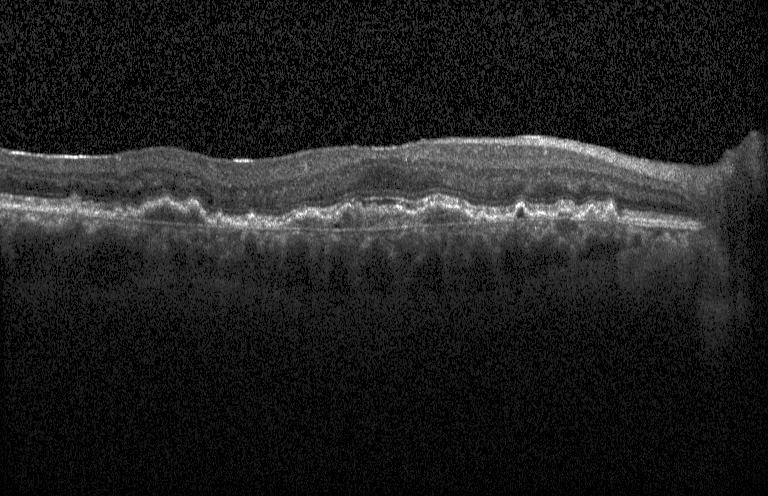
Spectral-domain OCT · Heidelberg Spectralis · retinal OCT cross-section · macular scan.
Diagnosis: choroidal neovascularization (CNV).